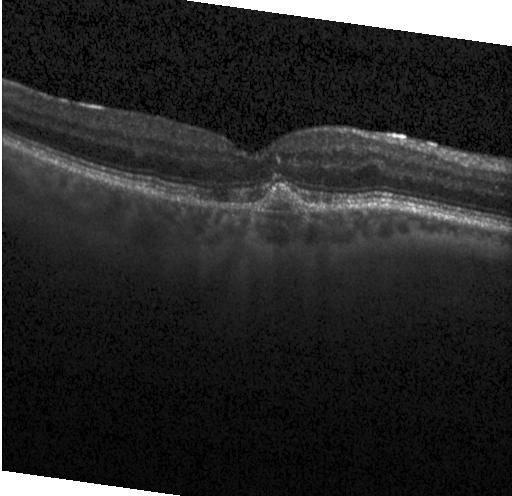

Spectral-domain optical coherence tomography, OCT line scan, fovea-centered.
Macular OCT: a choroidal neovascular membrane.